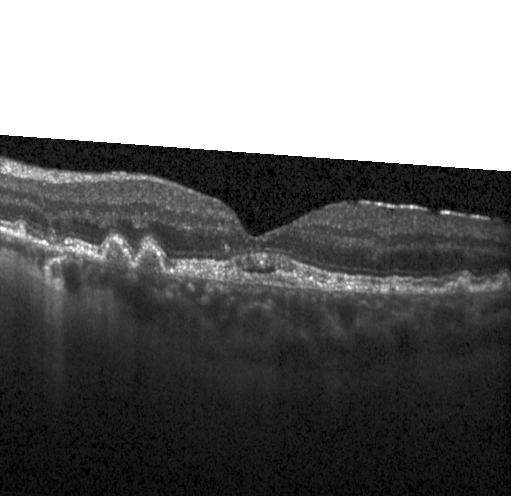 Assessment: a choroidal neovascular membrane.